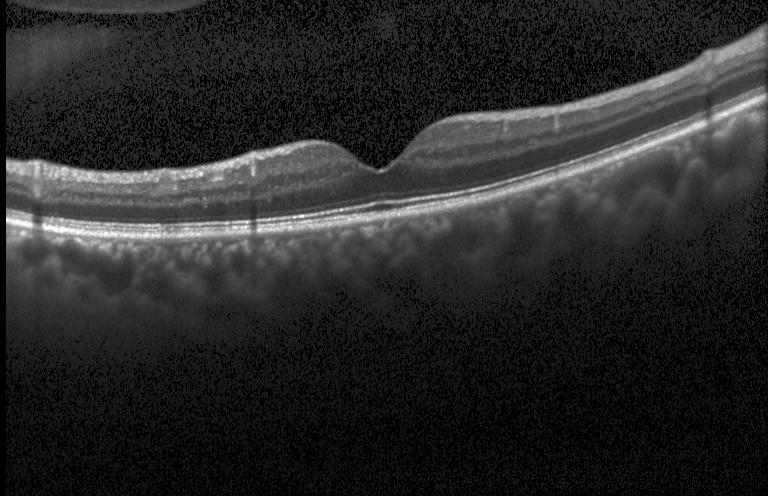
OCT finding: no choroidal neovascularization, no diabetic macular edema, and no drusen.